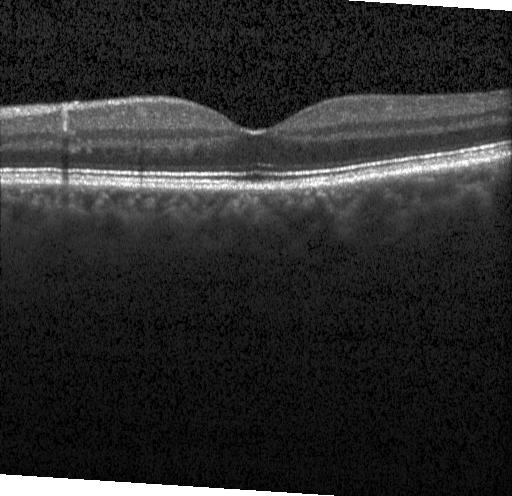

Spectral-domain OCT. Heidelberg Spectralis. Optical coherence tomography B-scan. Macular scan.
No CNV, no DME, and no drusen.